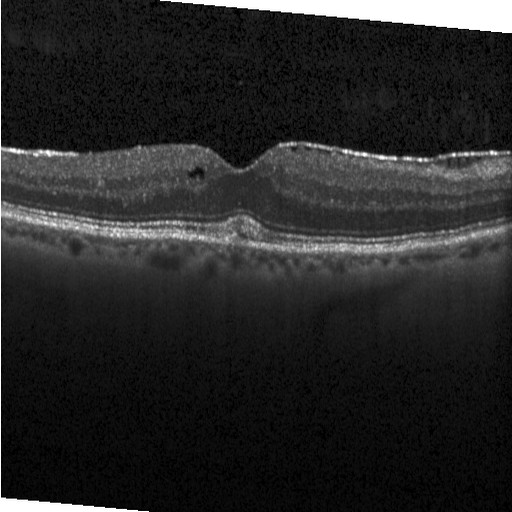 Heidelberg Spectralis OCT system; OCT line scan. The scan shows diabetic macular edema (DME).